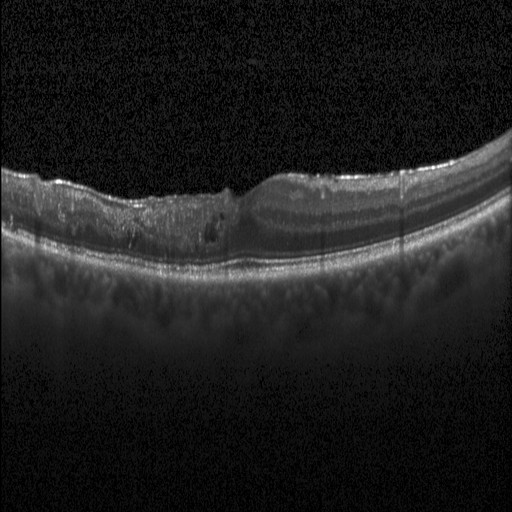 Retinal OCT B-scan
Impression: diabetic macular edema (DME).